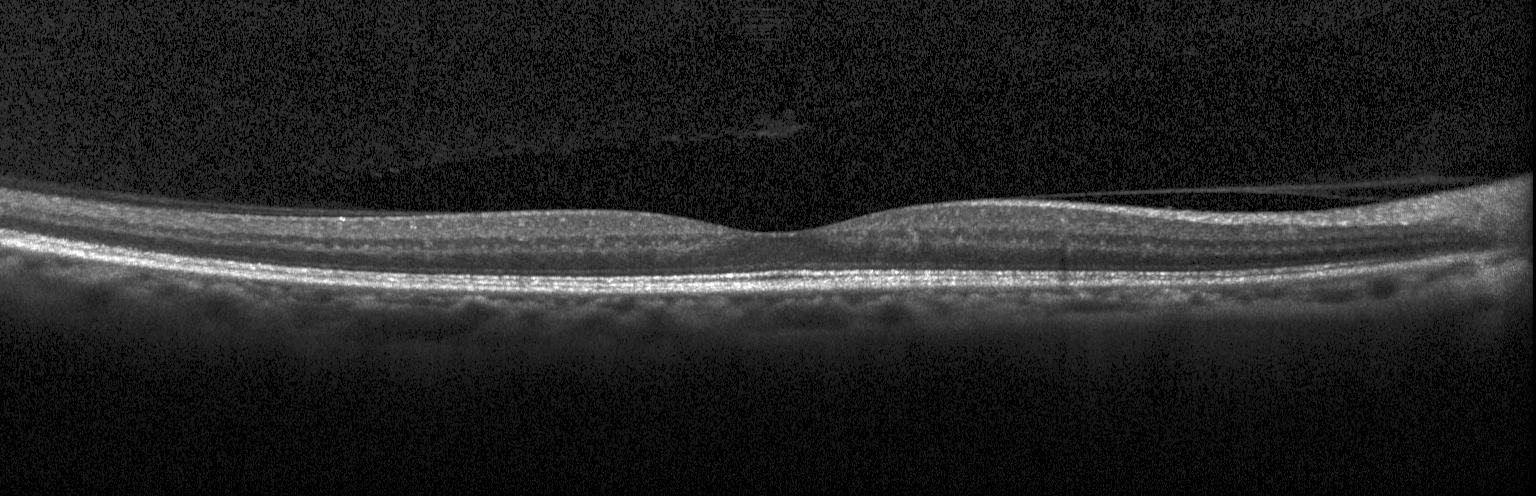

Dx: no choroidal neovascularization, no diabetic macular edema, and no drusen.